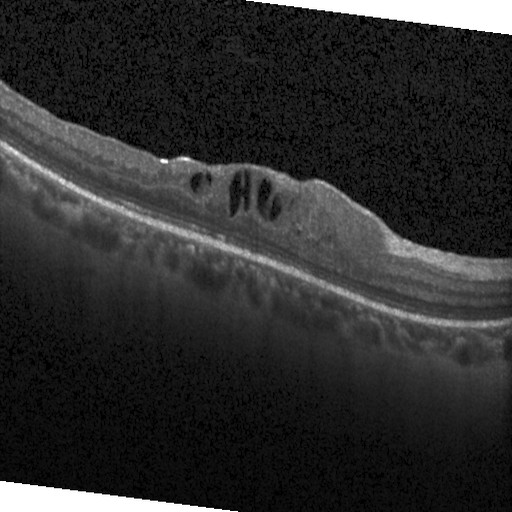

Spectral-domain optical coherence tomography. Retinal OCT cross-section. Fovea-centered — OCT finding: diabetic macular edema (DME).